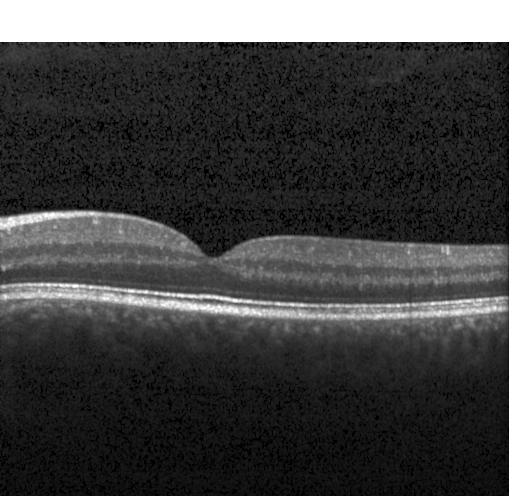

Impression: neither CNV, DME, nor drusen.